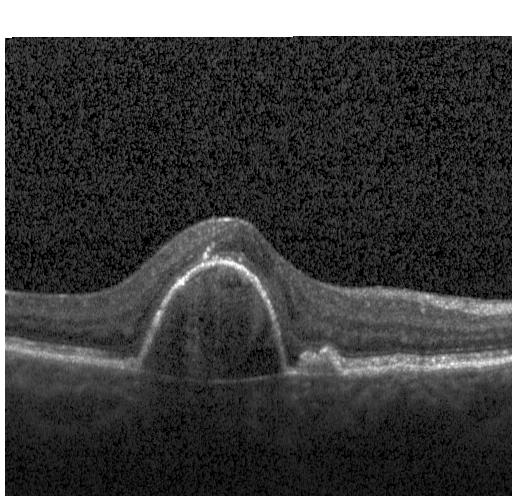

Finding: choroidal neovascularization (CNV).